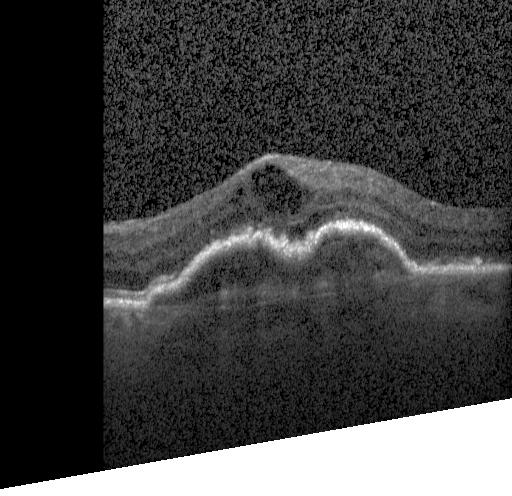 OCT finding: a choroidal neovascular membrane.